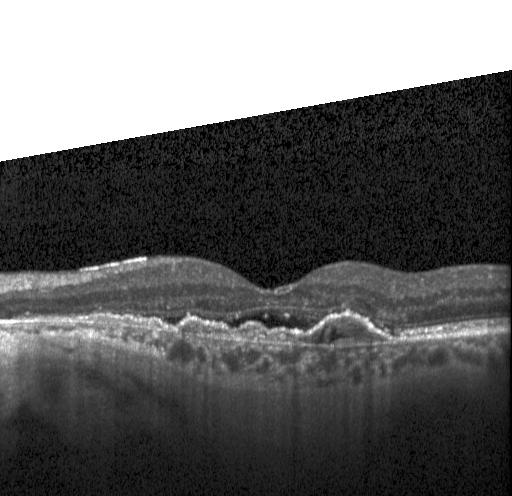

Fovea-centered · Heidelberg Spectralis · optical coherence tomography scan — Finding: CNV.